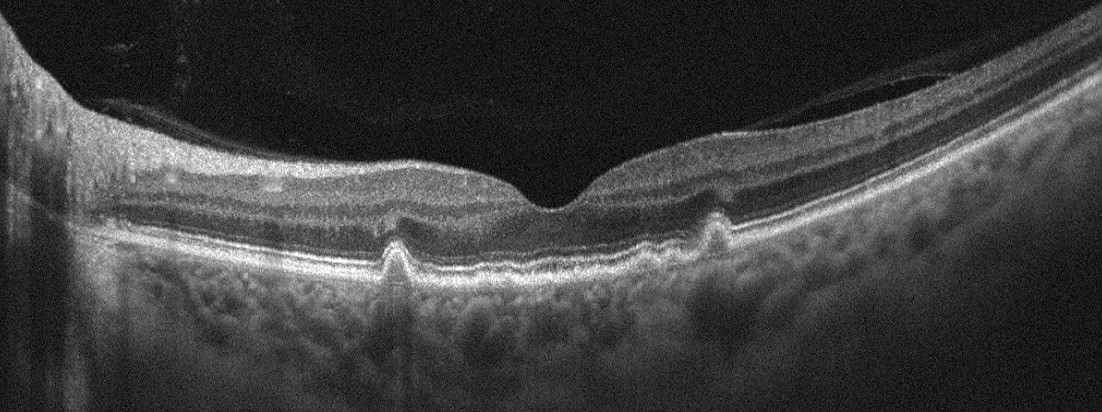

Optovue Avanti RTVue XR, retinal OCT cross-section — The scan shows age-related macular degeneration.